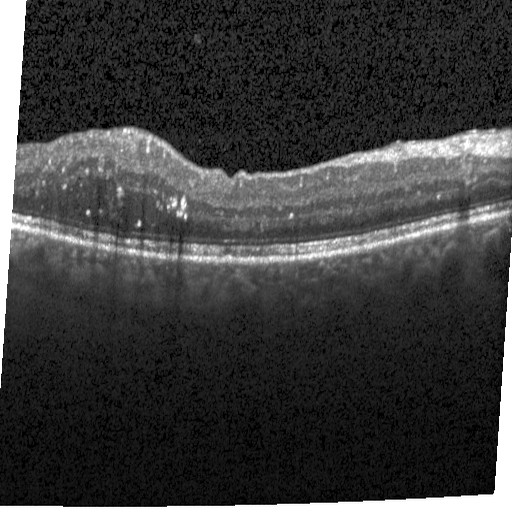 Spectral-domain optical coherence tomography. Retinal OCT cross-section — Diabetic macular edema (DME).